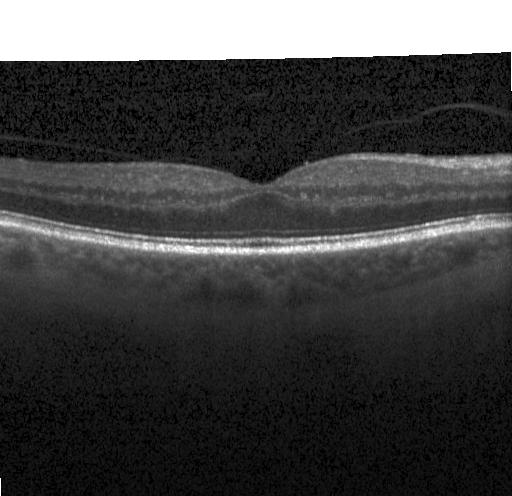
Impression: no evidence of choroidal neovascularization, diabetic macular edema, or drusen.